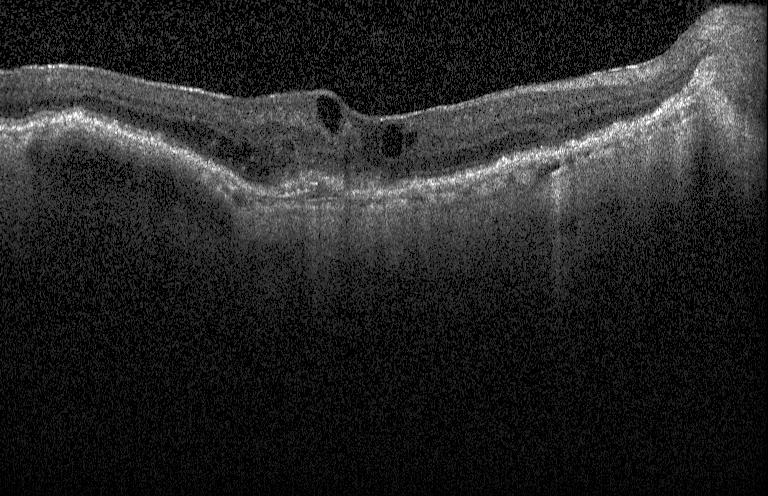
Diagnosis: choroidal neovascularization (CNV).